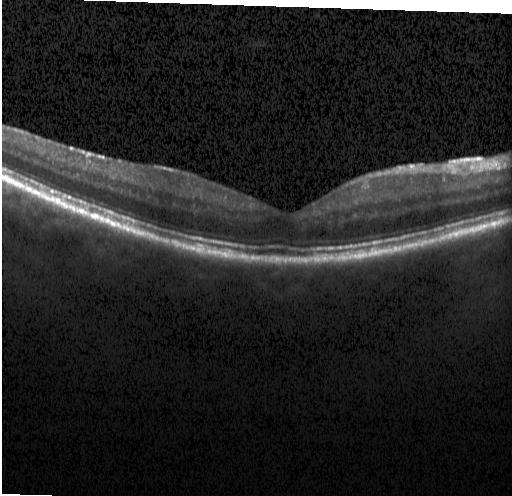
OCT B-scan showing no evidence of CNV, DME, or drusen.